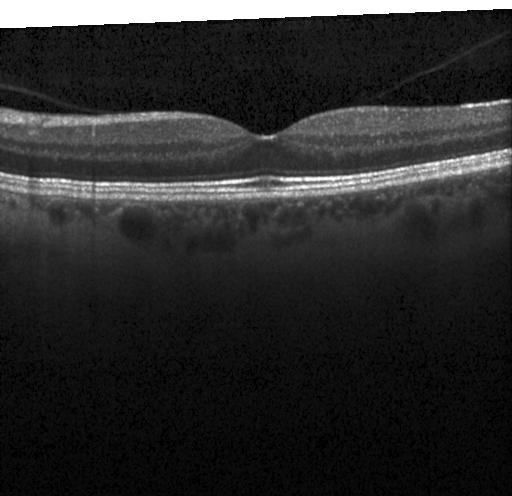

Finding: no evidence of CNV, DME, or drusen.